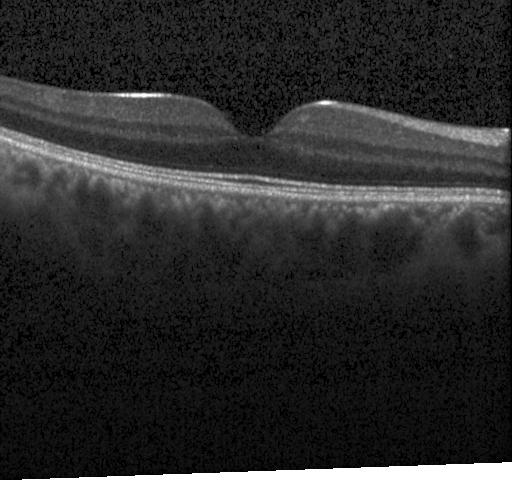

OCT B-scan showing no choroidal neovascularization, no diabetic macular edema, and no drusen.